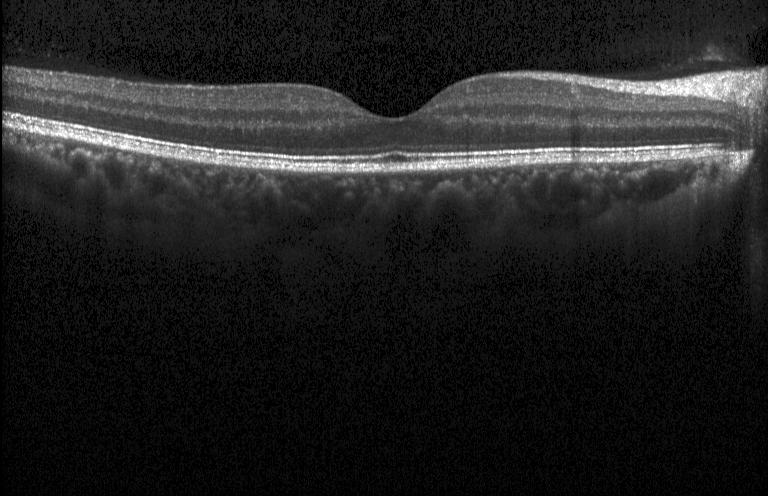 Impression: neither choroidal neovascularization, diabetic macular edema, nor drusen.